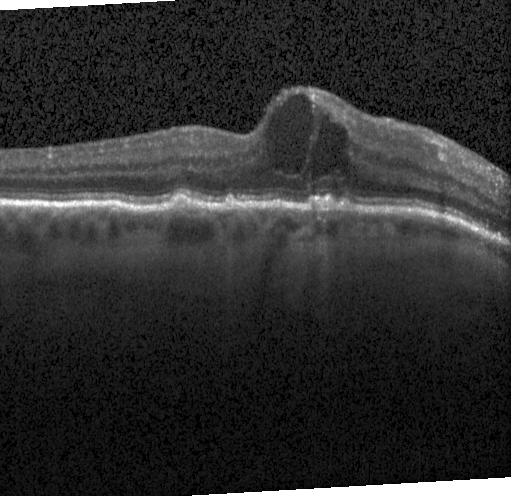

Assessment: a choroidal neovascular membrane.